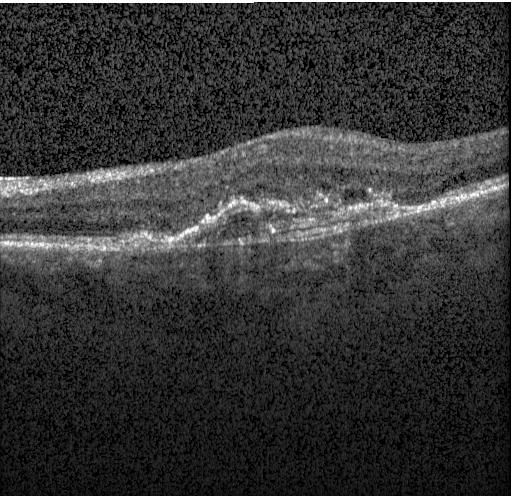 OCT B-scan, spectral-domain optical coherence tomography.
Impression: choroidal neovascularization.